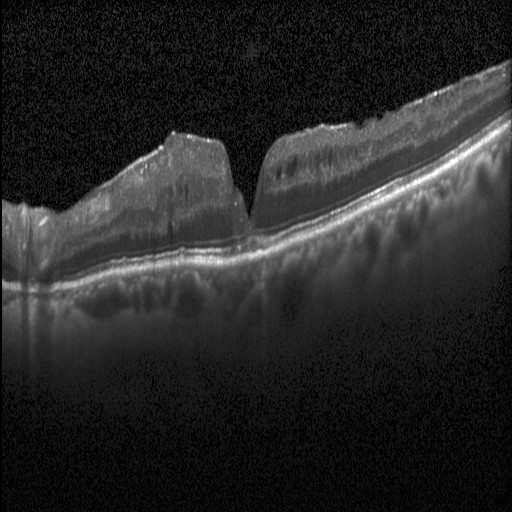
OCT line scan; macular scan. This B-scan demonstrates DME.